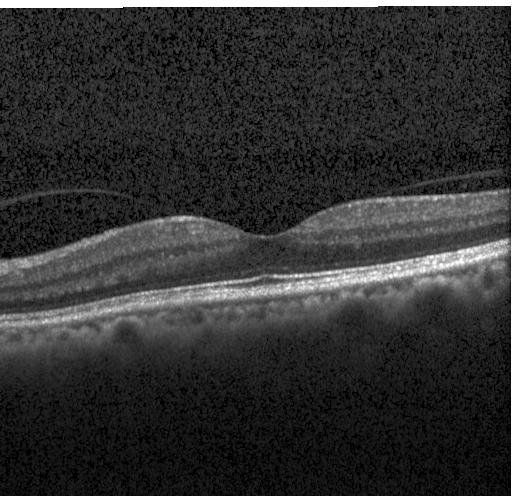
OCT line scan — Diagnosis: no CNV, no DME, and no drusen.